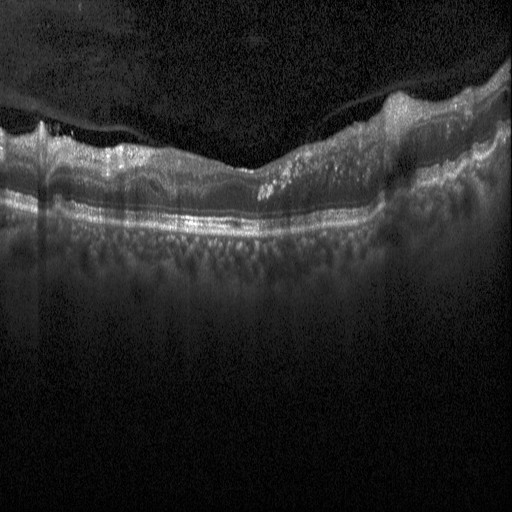 Heidelberg Spectralis OCT system. Macular scan. Retinal OCT B-scan
Assessment: DME.